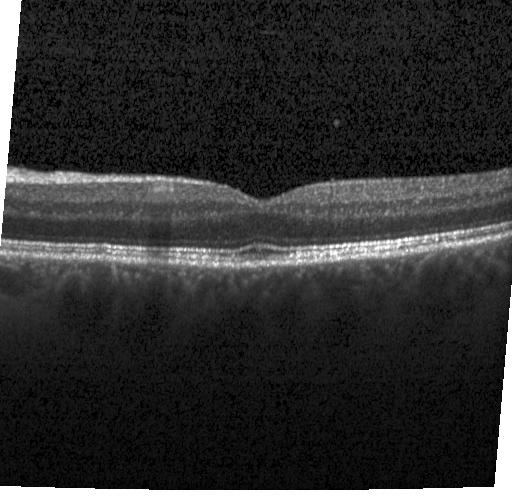 This B-scan demonstrates no evidence of choroidal neovascularization, diabetic macular edema, or drusen.